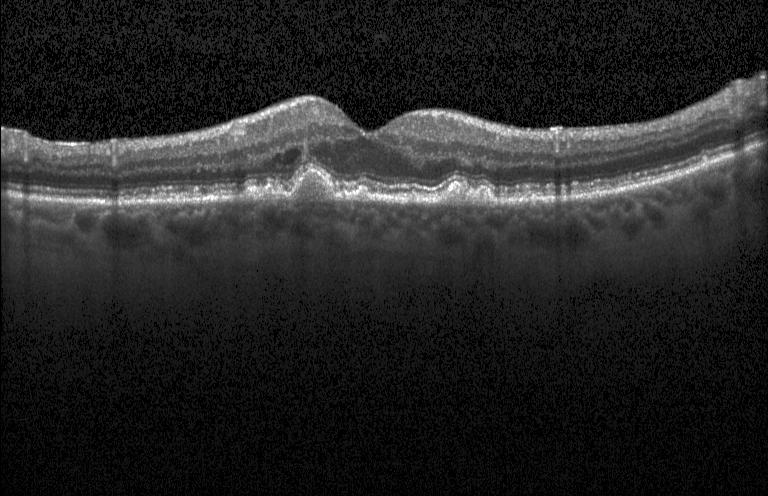

SD-OCT. Acquired on a Heidelberg Spectralis. Retinal OCT cross-section — Dx: sub-RPE drusenoid deposits.